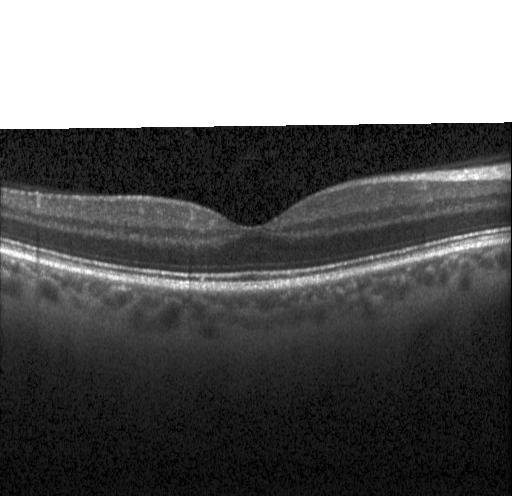
Fovea-centered; spectral-domain OCT; instrument: Heidelberg Spectralis; OCT B-scan. Macular OCT: neither choroidal neovascularization, diabetic macular edema, nor drusen.